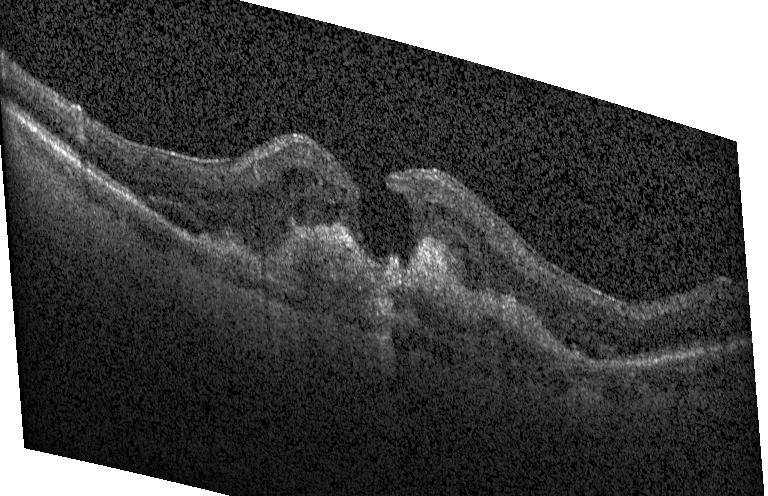
Optical coherence tomography B-scan, SD-OCT.
Diagnosis: a choroidal neovascular membrane.